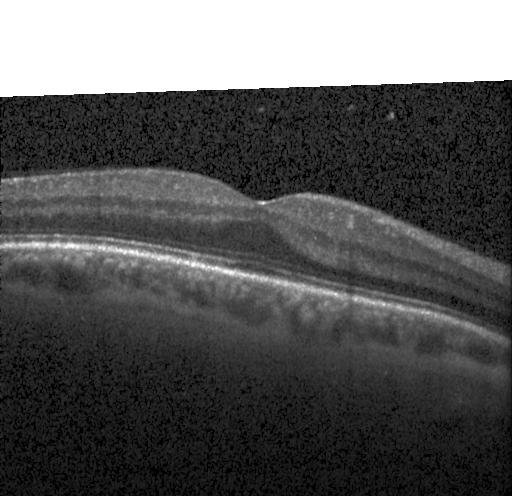
Retinal OCT cross-section; SD-OCT — Impression: neither choroidal neovascularization, diabetic macular edema, nor drusen.